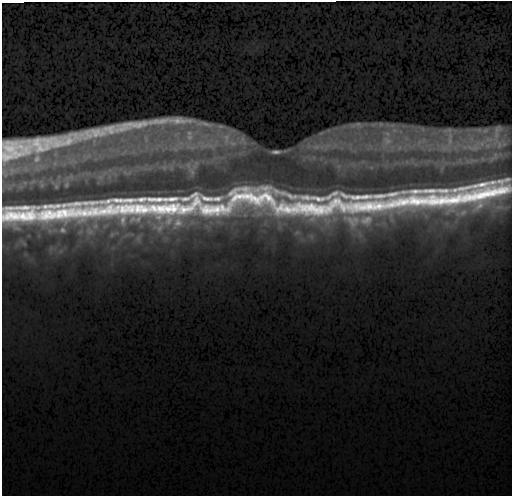
Finding: sub-RPE drusenoid deposits.